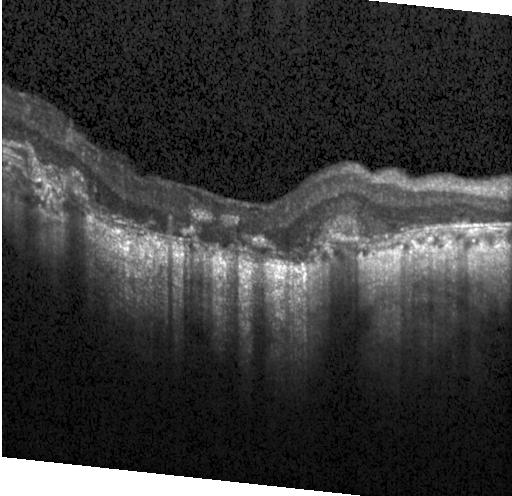

Heidelberg Spectralis OCT system. Retinal OCT B-scan
Impression: choroidal neovascularization (CNV).